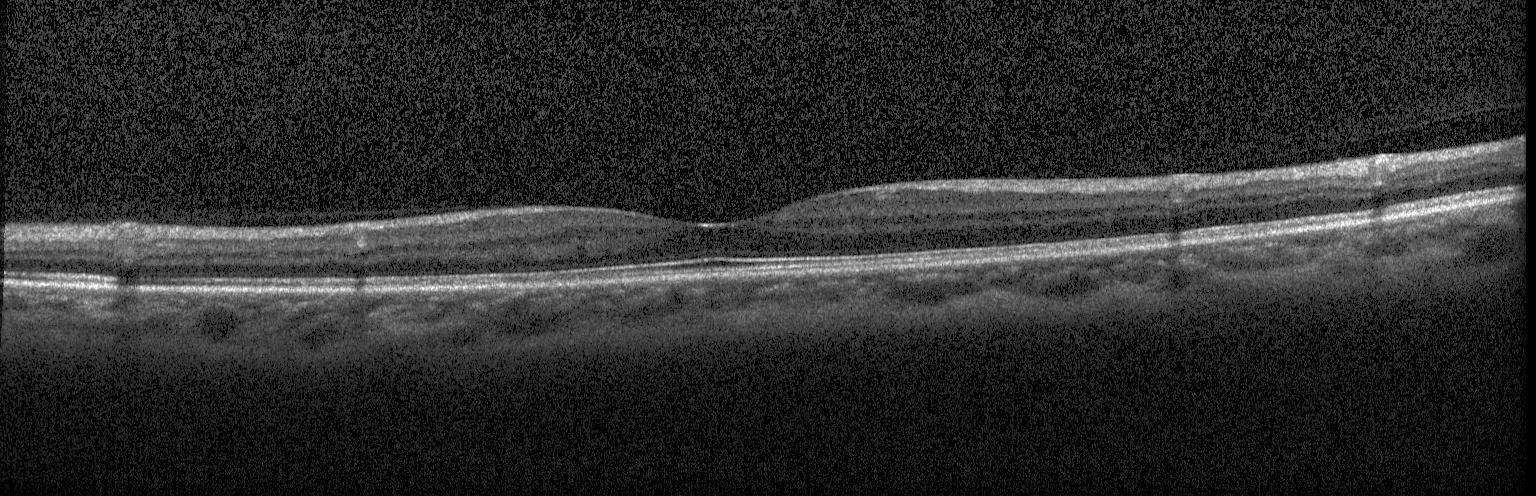 No choroidal neovascularization, no diabetic macular edema, and no drusen.